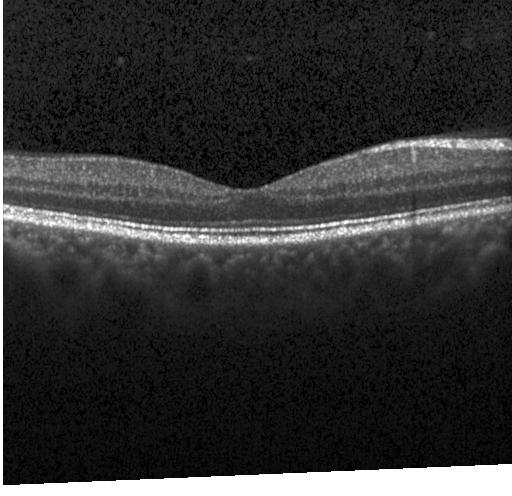 Spectral-domain OCT; instrument: Heidelberg Spectralis; OCT B-scan; centered on the fovea — Diagnosis: no choroidal neovascularization, no diabetic macular edema, and no drusen.